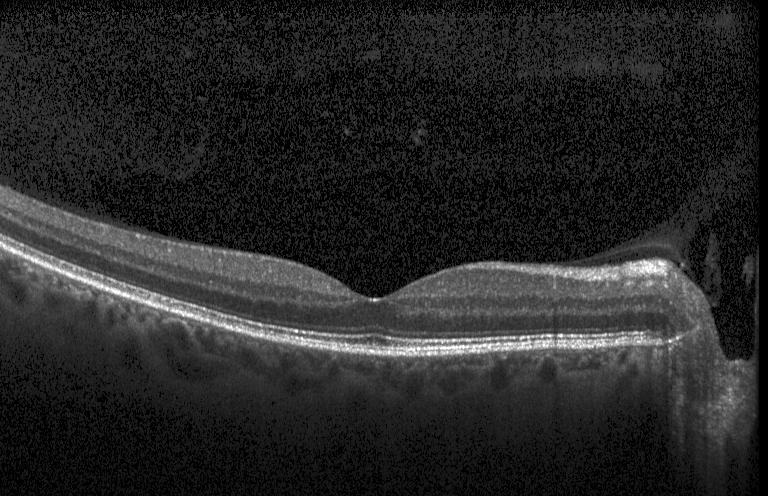
Fovea-centered, Heidelberg Spectralis, retinal OCT cross-section.
OCT finding: no evidence of choroidal neovascularization, diabetic macular edema, or drusen.